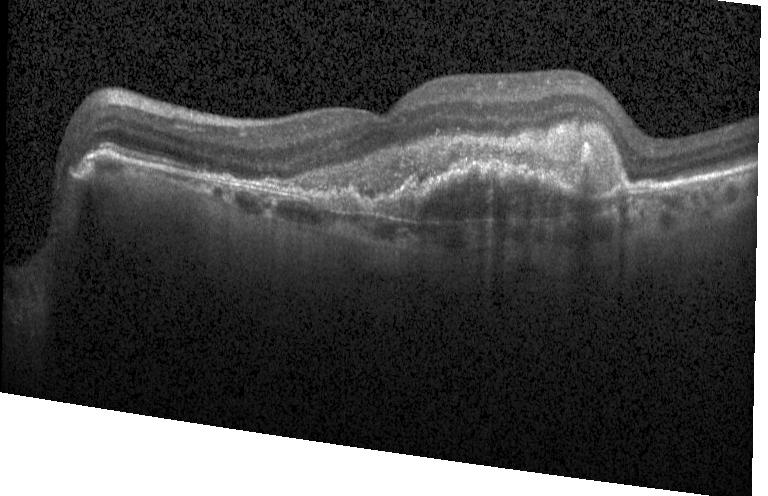
OCT B-scan.
Diagnosis: choroidal neovascularization (CNV).